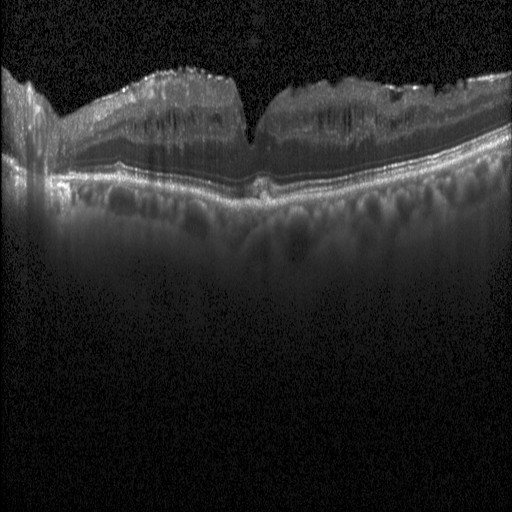
SD-OCT, retinal OCT cross-section, instrument: Heidelberg Spectralis. This B-scan demonstrates diabetic macular edema.